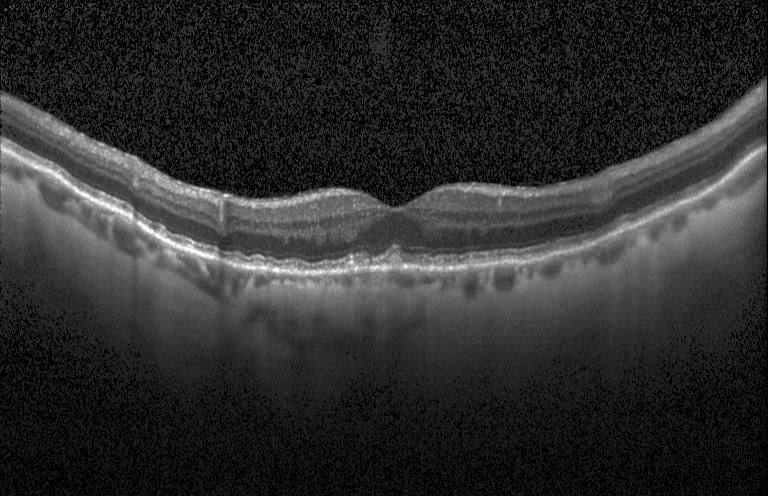 Optical coherence tomography scan.
Diagnosis: sub-RPE drusenoid deposits.